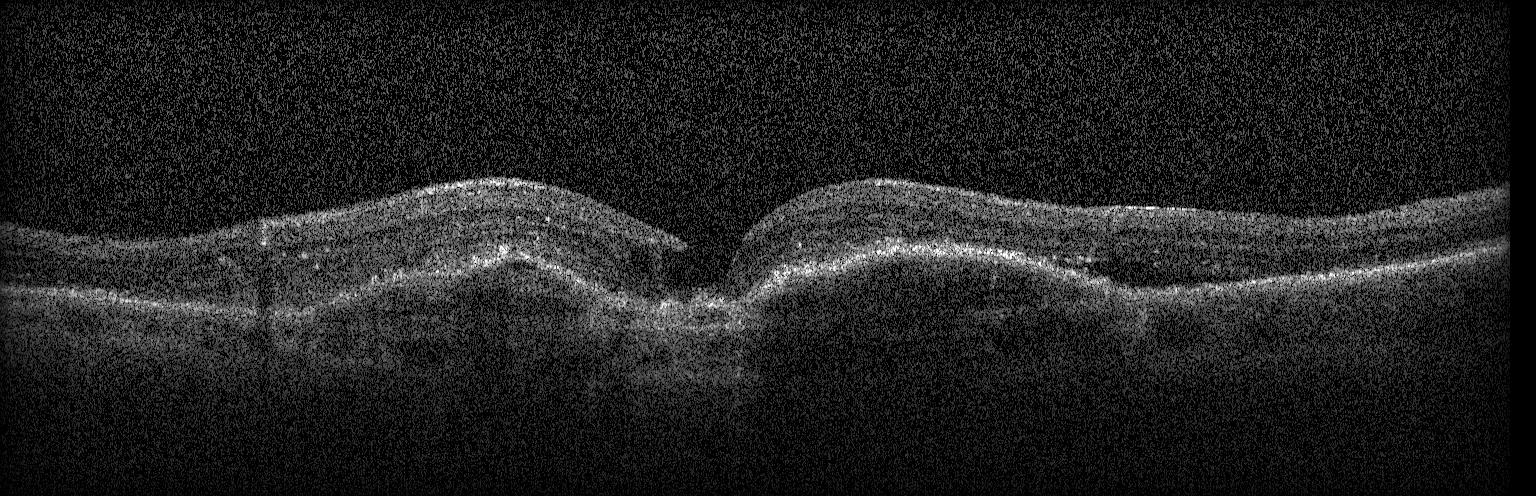

Acquired on a Heidelberg Spectralis · spectral-domain OCT · centered on the fovea · retinal OCT B-scan. Impression: a choroidal neovascular membrane.